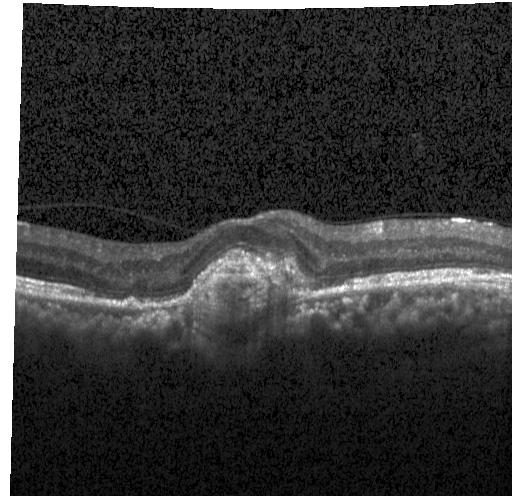
OCT B-scan showing a choroidal neovascular membrane.